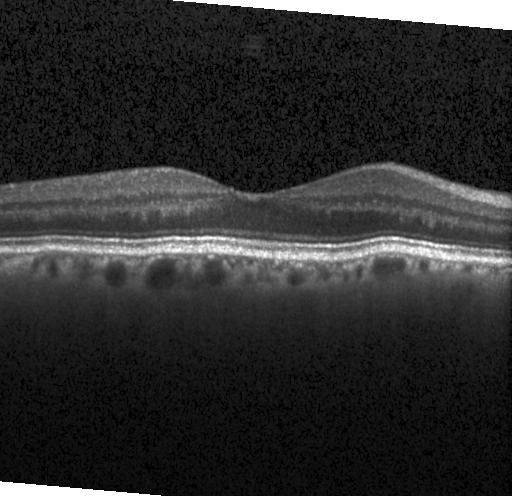
Impression: no CNV, DME, or drusen.